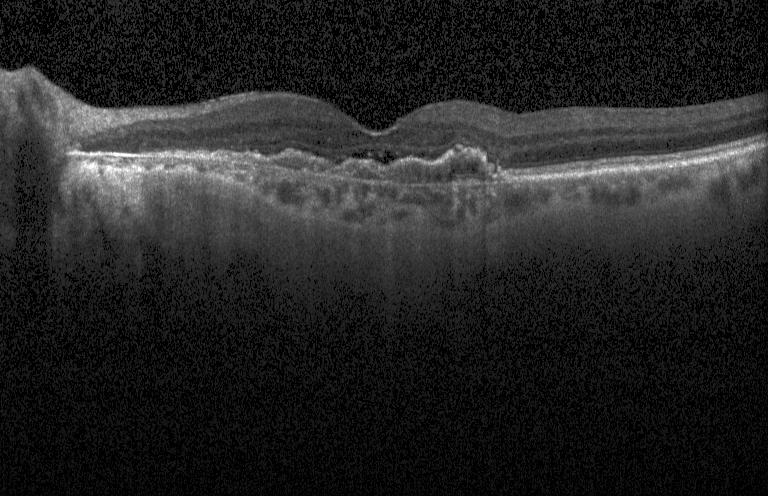

OCT line scan; macular scan; Heidelberg Spectralis
Impression: CNV.